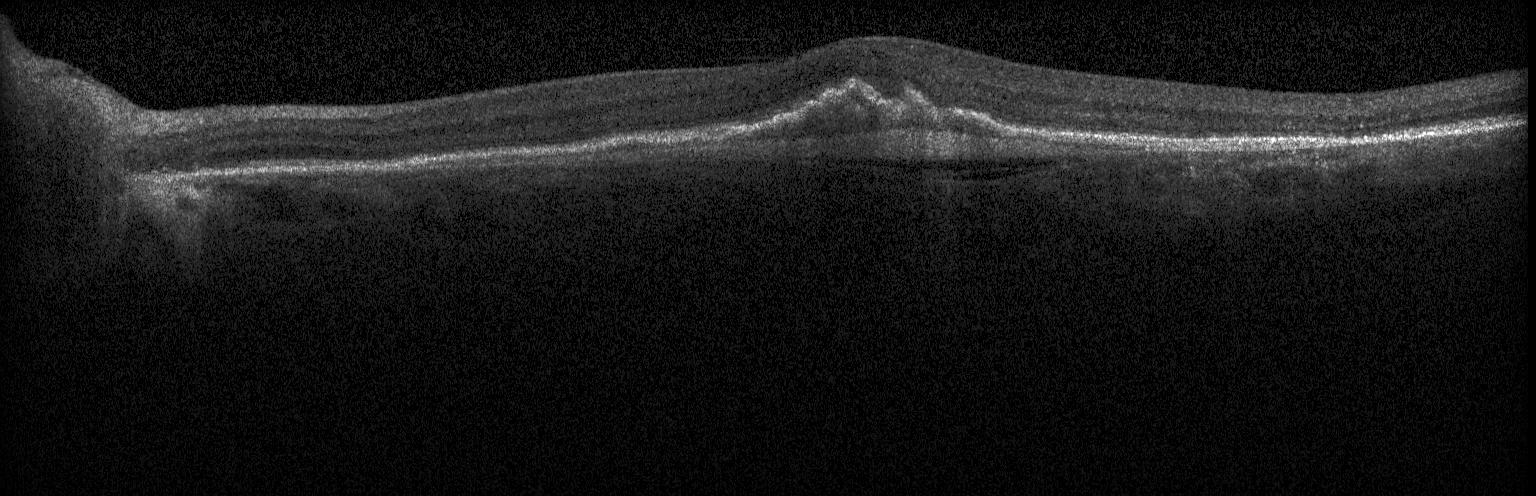 Macular OCT: a choroidal neovascular membrane.